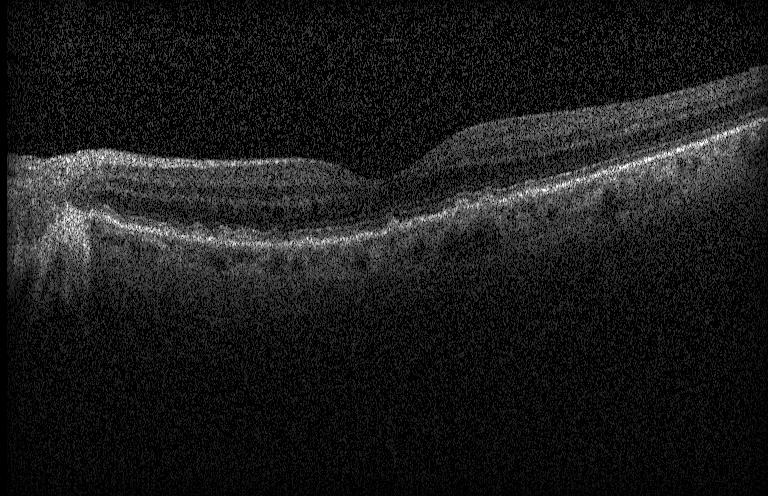
Heidelberg Spectralis OCT system · spectral-domain OCT · retinal OCT B-scan — The scan shows sub-RPE drusenoid deposits.